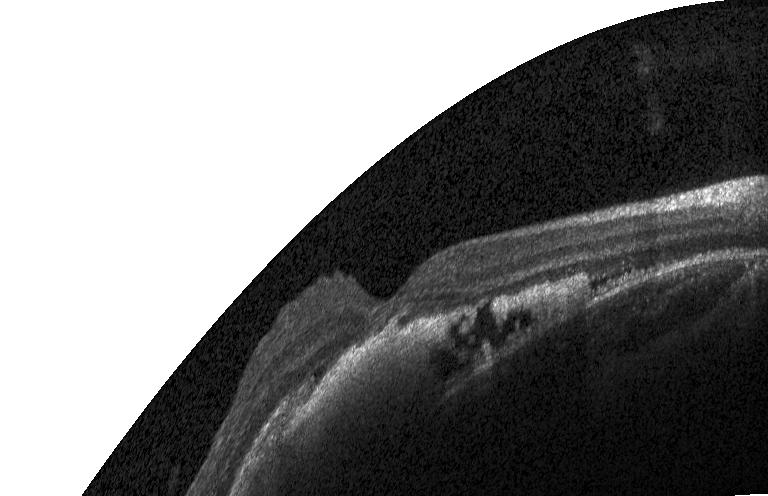 OCT B-scan showing a choroidal neovascular membrane.